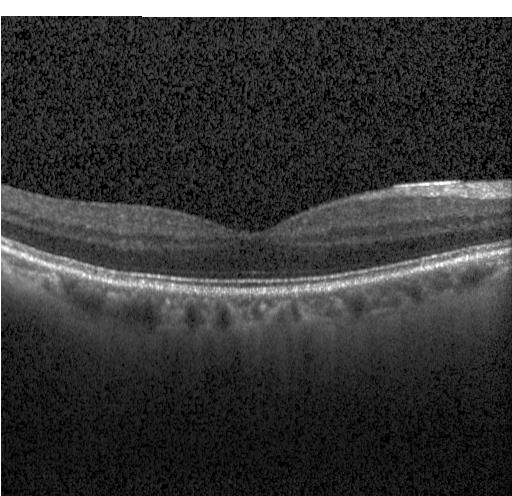

Centered on the fovea · acquired on a Heidelberg Spectralis · retinal OCT B-scan · SD-OCT.
The scan shows neither choroidal neovascularization, diabetic macular edema, nor drusen.